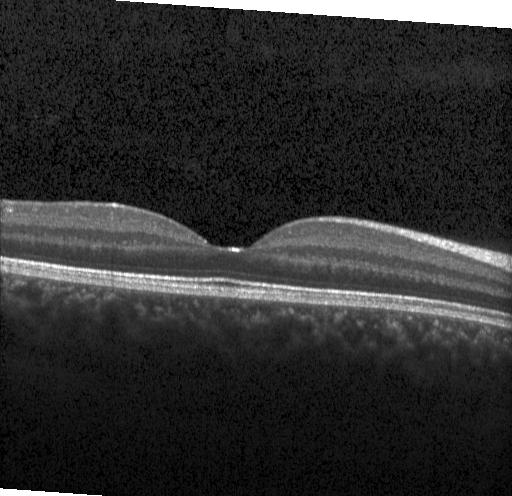 Optical coherence tomography B-scan. Centered on the fovea — OCT finding: no choroidal neovascularization, no diabetic macular edema, and no drusen.